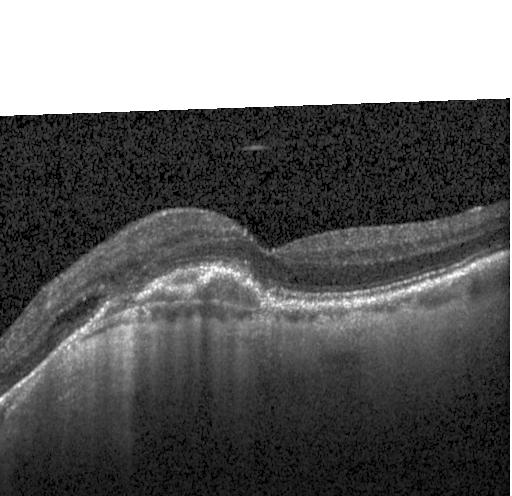 Macular OCT demonstrating choroidal neovascularization (CNV).